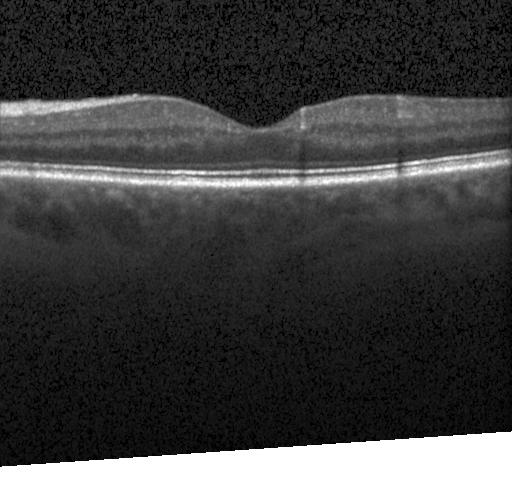

OCT line scan; macular scan
Dx: no choroidal neovascularization, no diabetic macular edema, and no drusen.